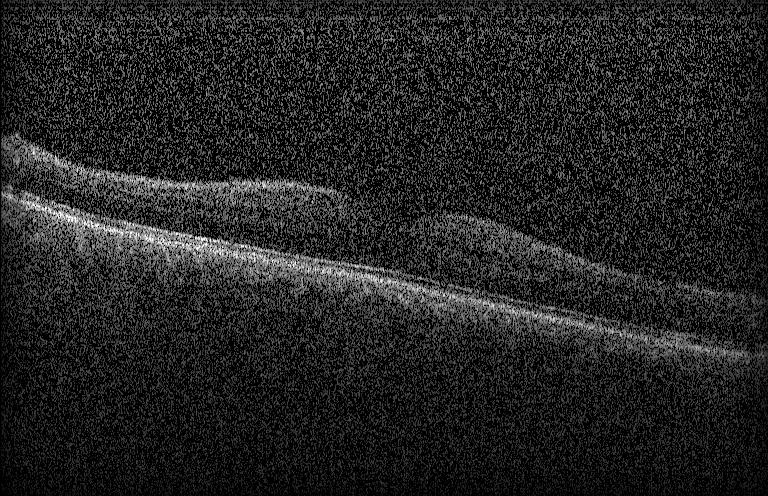
Macular OCT demonstrating no evidence of choroidal neovascularization, diabetic macular edema, or drusen.